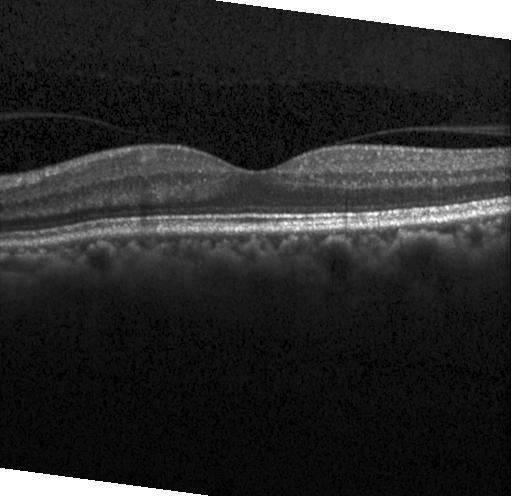 Spectral-domain optical coherence tomography; macular scan; OCT B-scan; Heidelberg Spectralis OCT system. The scan shows no evidence of choroidal neovascularization, diabetic macular edema, or drusen.